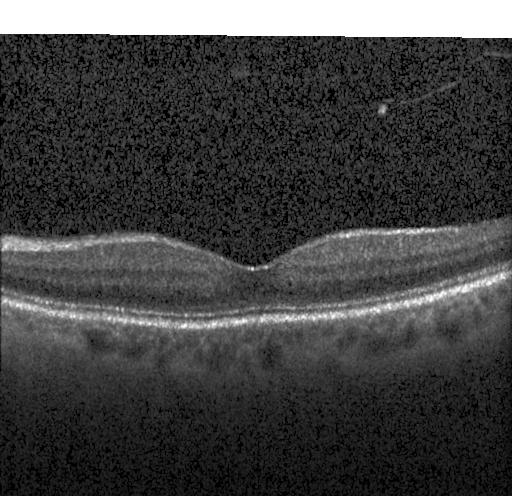 Dx: no choroidal neovascularization, diabetic macular edema, or drusen.